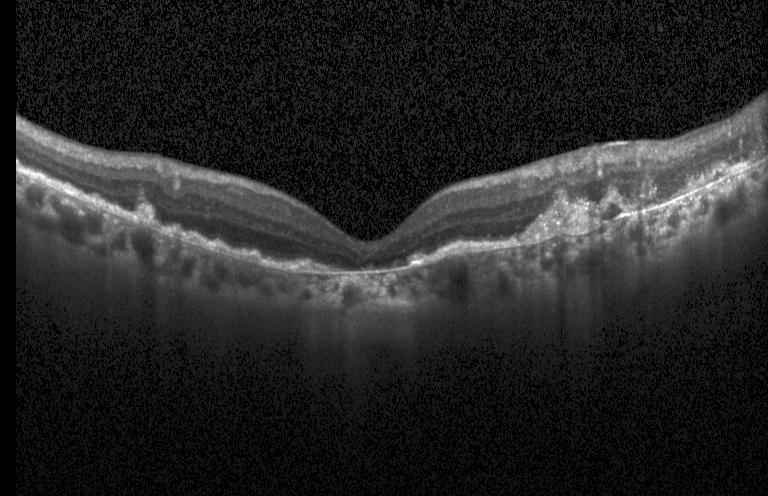
Heidelberg Spectralis OCT system · SD-OCT · retinal OCT B-scan · through the macula.
Finding: choroidal neovascularization (CNV).